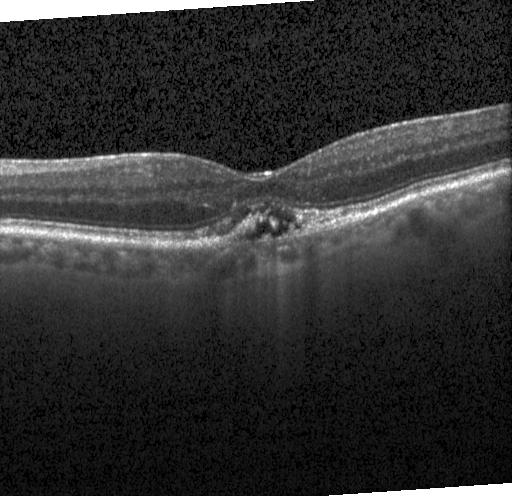
Diagnosis: CNV.